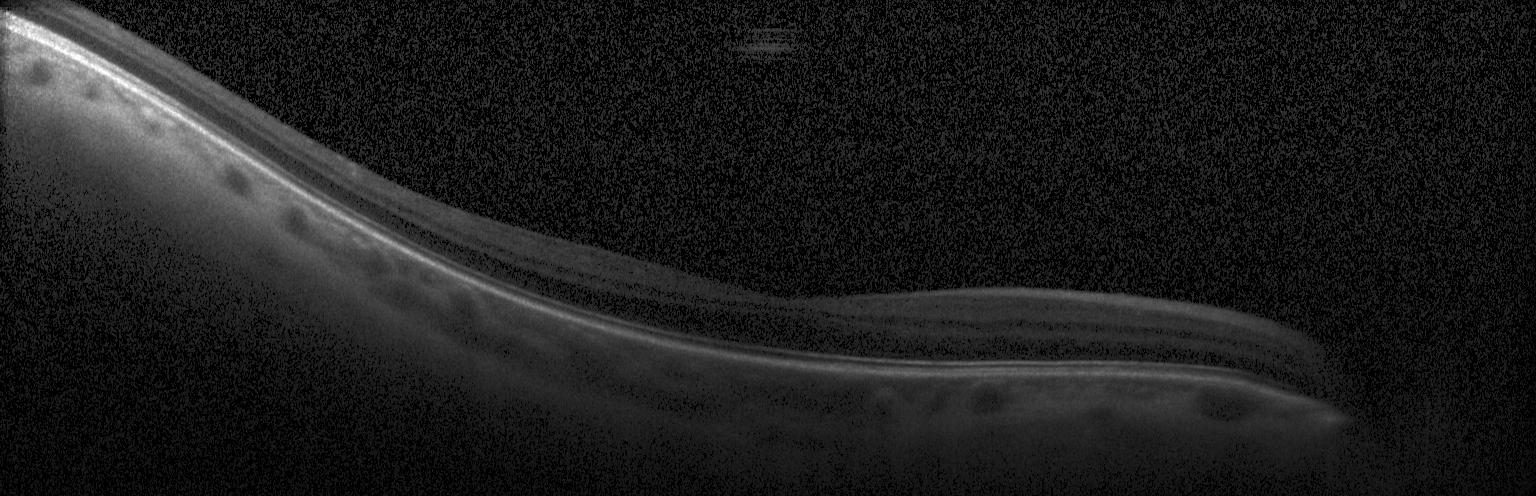 Macular OCT: no choroidal neovascularization, no diabetic macular edema, and no drusen.